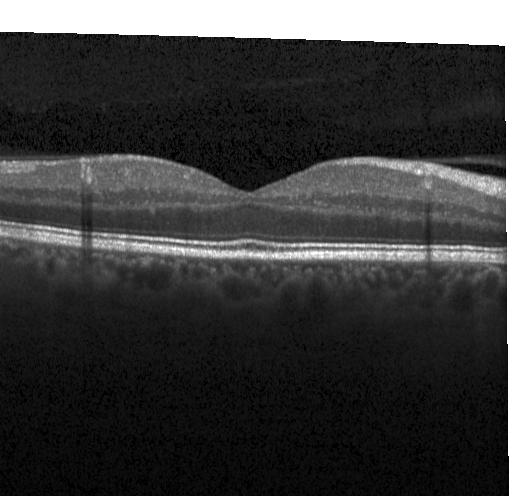 Macular scan · instrument: Heidelberg Spectralis · optical coherence tomography B-scan.
Finding: neither choroidal neovascularization, diabetic macular edema, nor drusen.